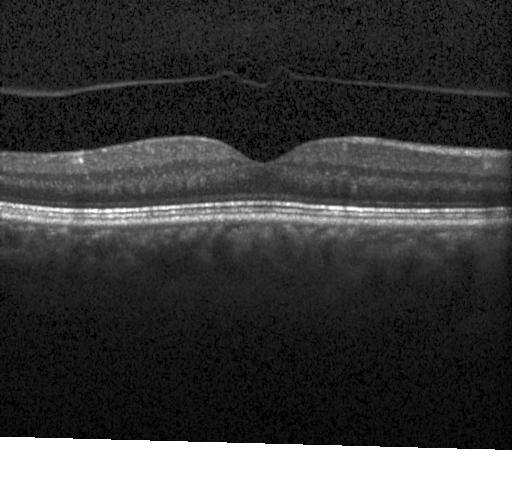

OCT finding: neither choroidal neovascularization, diabetic macular edema, nor drusen.